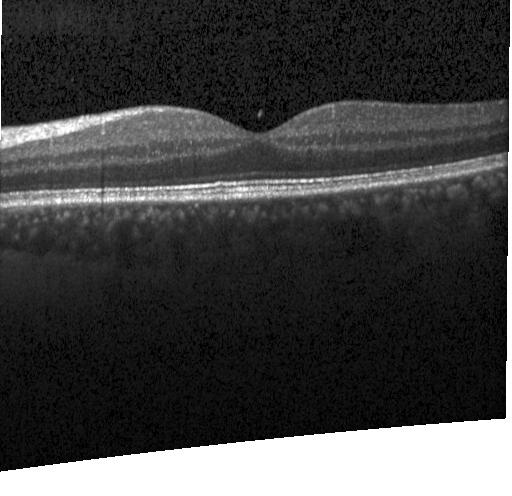

Heidelberg Spectralis OCT system, horizontal scan through the fovea, OCT B-scan
This B-scan demonstrates no evidence of choroidal neovascularization, diabetic macular edema, or drusen.